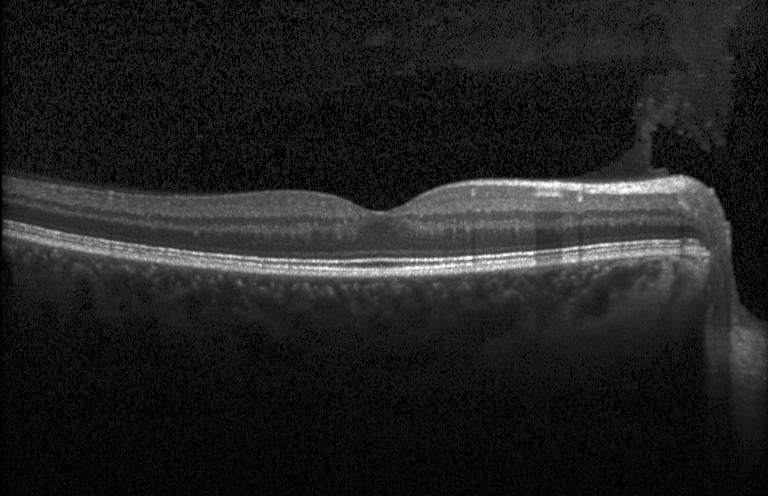
OCT B-scan.
OCT finding: no choroidal neovascularization, no diabetic macular edema, and no drusen.